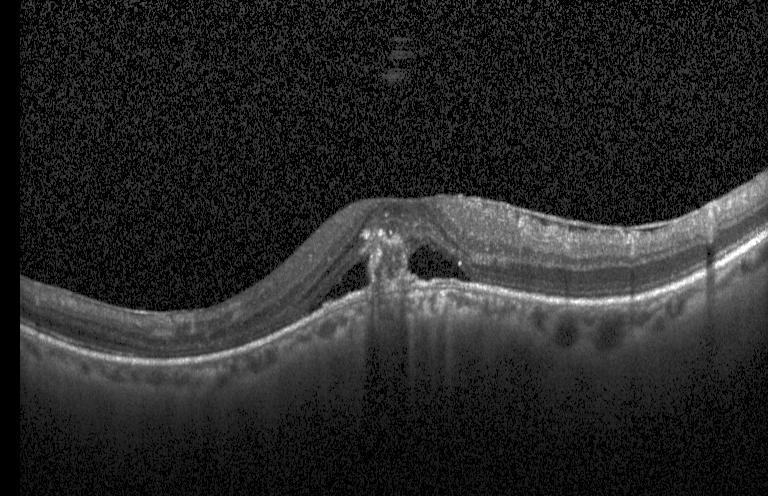 Retinal OCT cross-section showing a choroidal neovascular membrane.